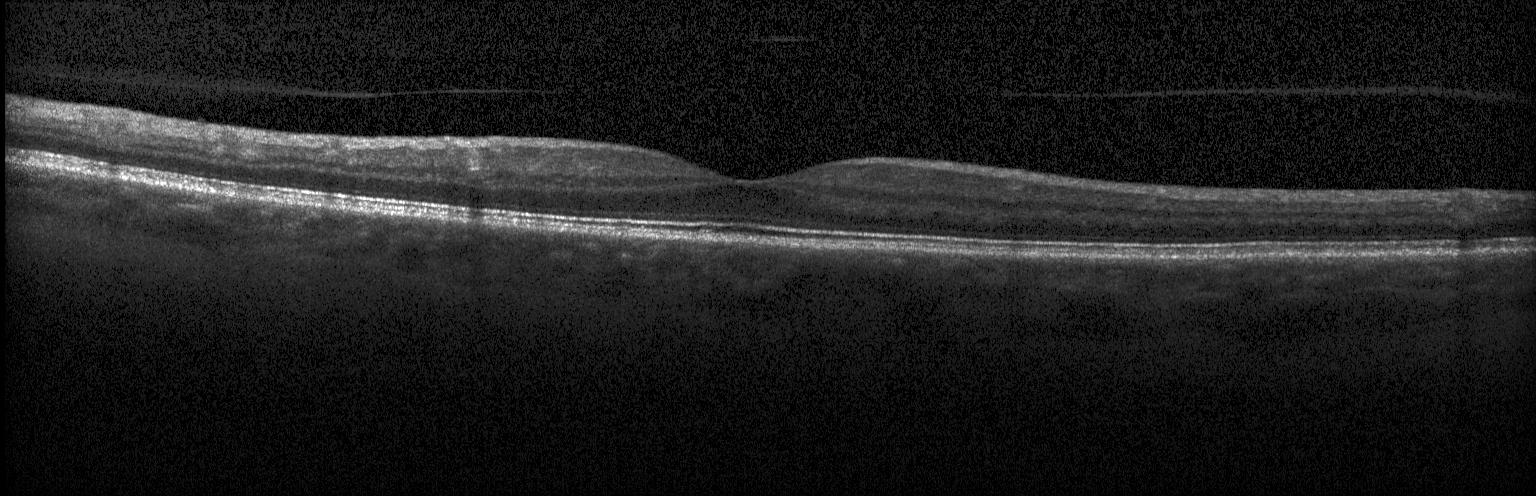 Impression: no choroidal neovascularization, diabetic macular edema, or drusen.